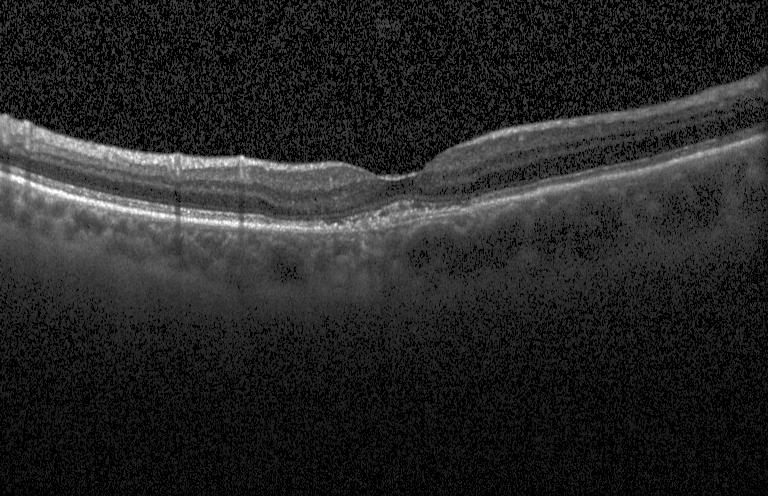 Finding: choroidal neovascularization (CNV).